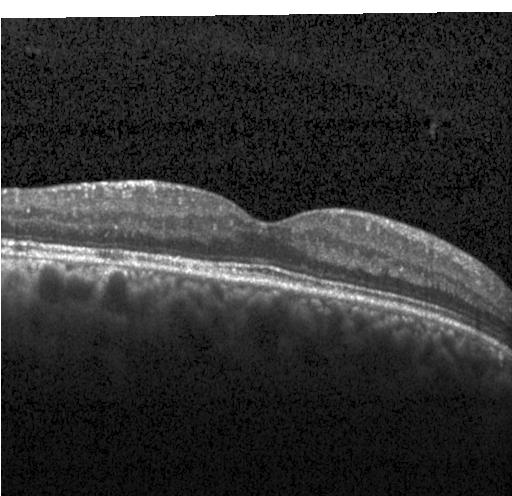

Impression: no choroidal neovascularization, no diabetic macular edema, and no drusen.